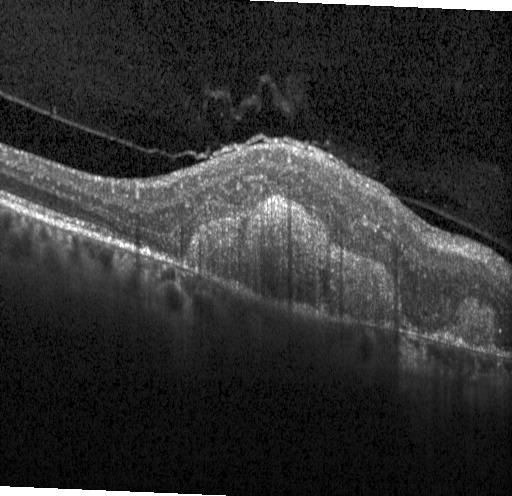
Impression: CNV.